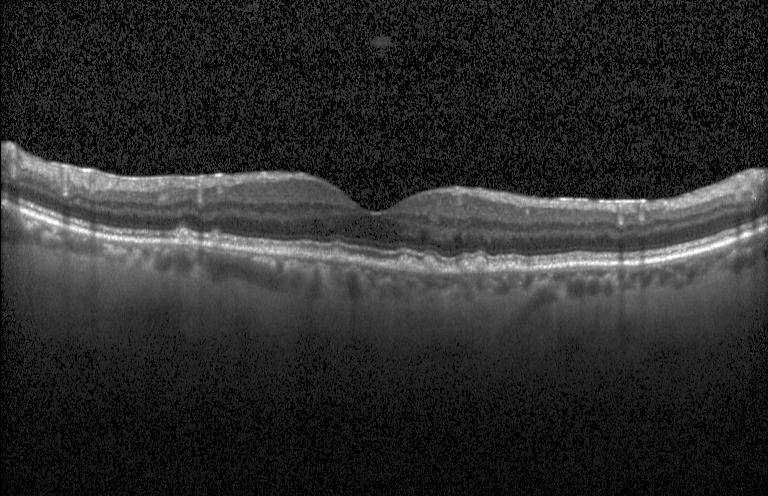

OCT line scan. Heidelberg Spectralis OCT system. SD-OCT. Through the macula
Finding: multiple drusen.